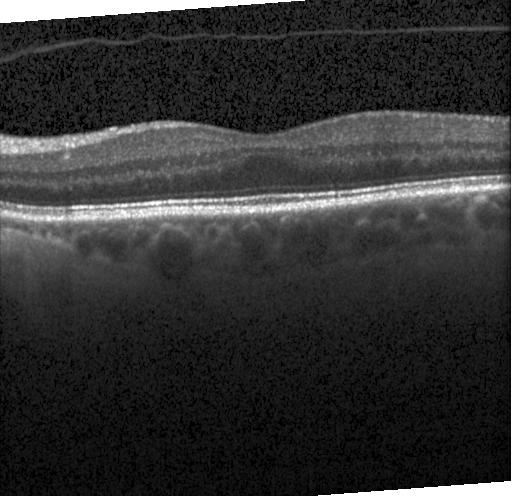 Fovea-centered; OCT B-scan; Heidelberg Spectralis OCT system
Impression: no CNV, no DME, and no drusen.